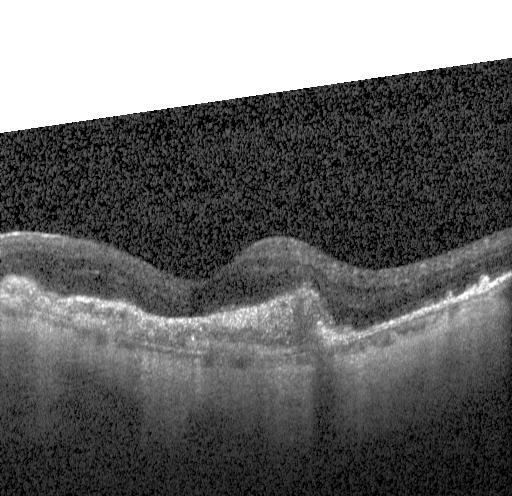
Spectral-domain OCT B-scan: CNV.